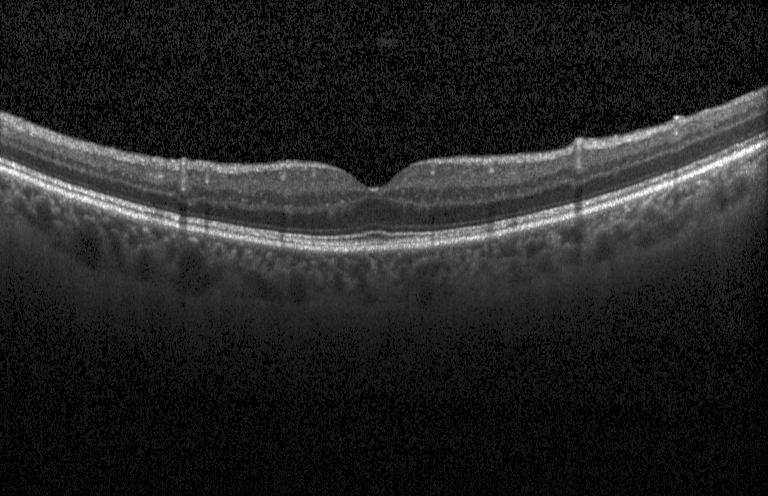
OCT scan showing no choroidal neovascularization, diabetic macular edema, or drusen.